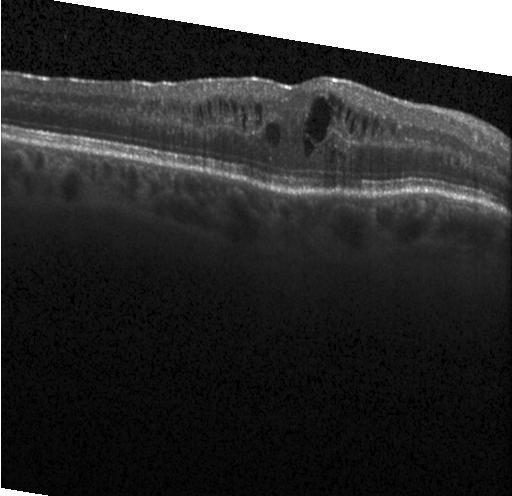 Optical coherence tomography B-scan. Centered on the fovea. Spectral-domain OCT
Impression: diabetic macular edema.